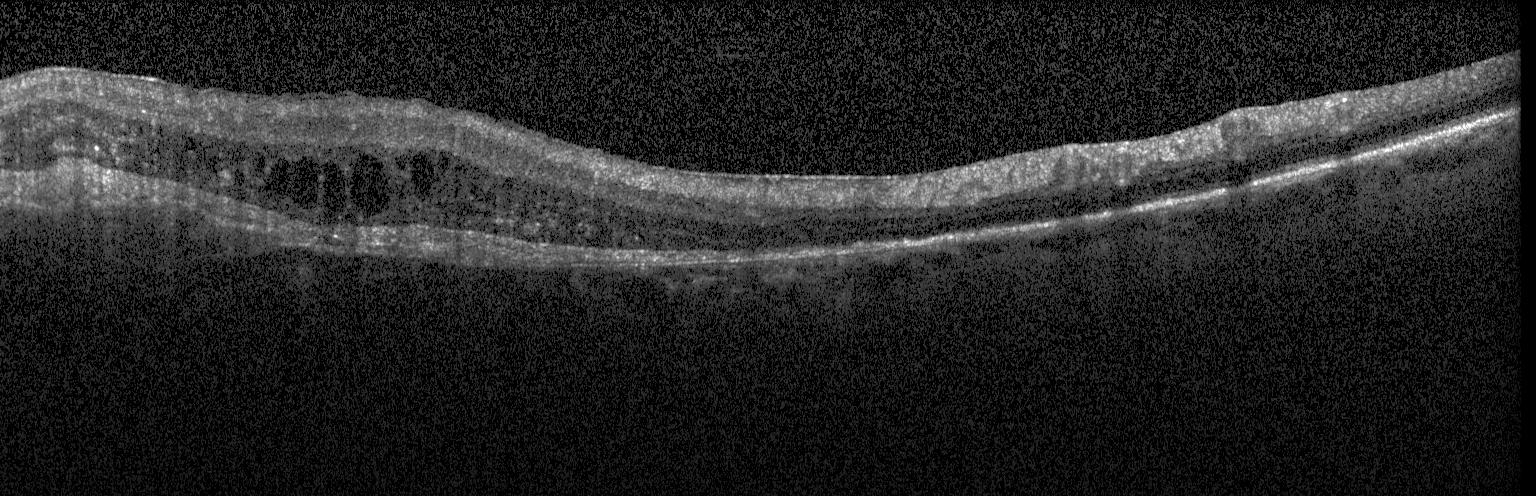
Retinal OCT cross-section
Impression: choroidal neovascularization.